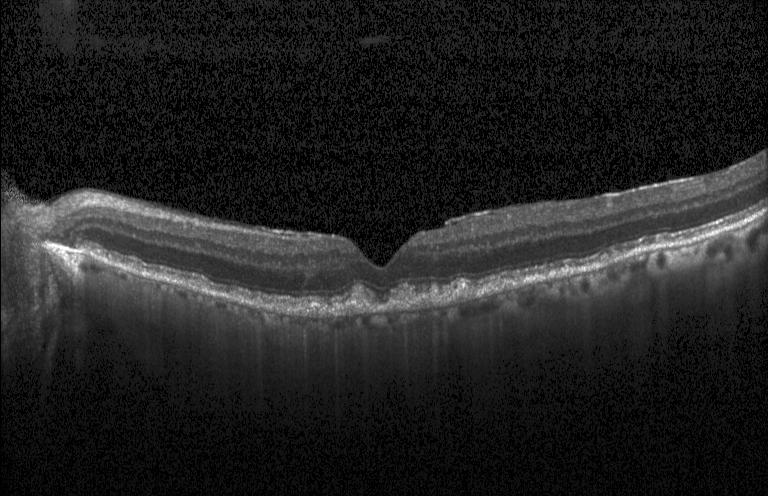
Instrument: Heidelberg Spectralis, spectral-domain OCT, retinal OCT cross-section
OCT finding: drusen.